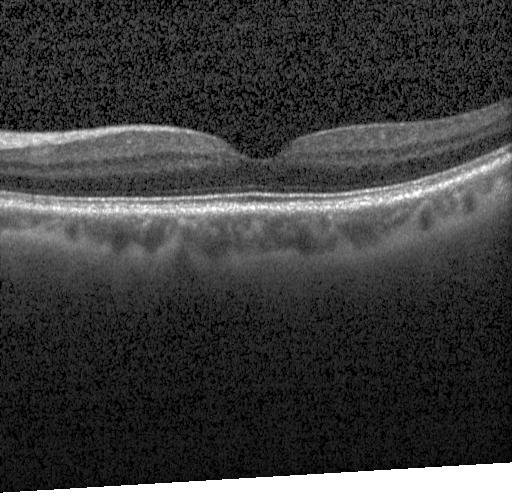
OCT B-scan · spectral-domain OCT · Heidelberg Spectralis OCT system. OCT finding: neither choroidal neovascularization, diabetic macular edema, nor drusen.